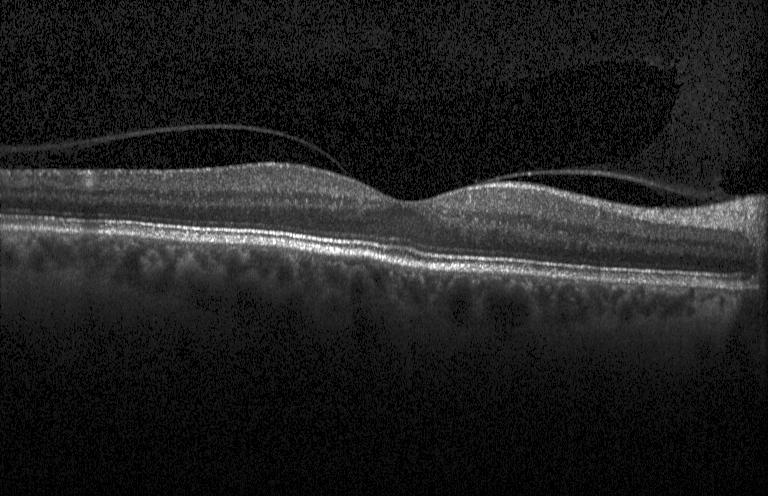
Macular OCT: no CNV, no DME, and no drusen.